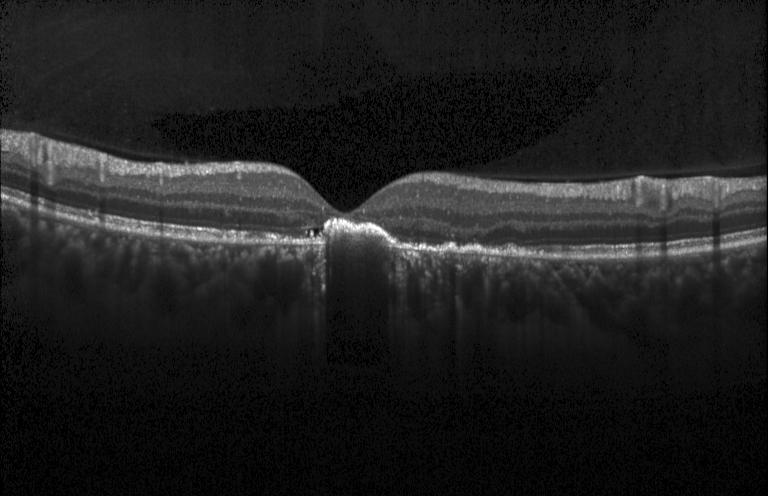 Finding: a choroidal neovascular membrane.